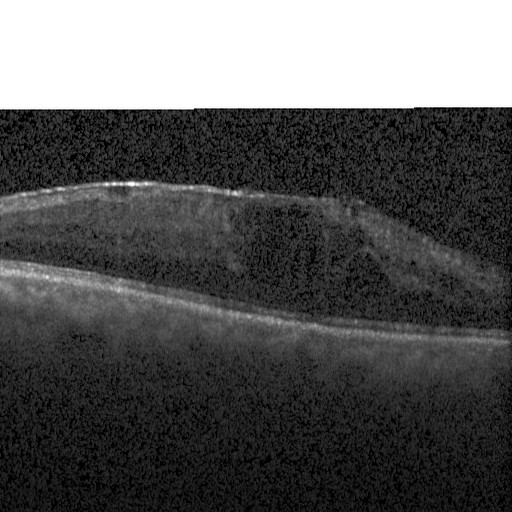
Retinal OCT B-scan.
Finding: diabetic macular edema.